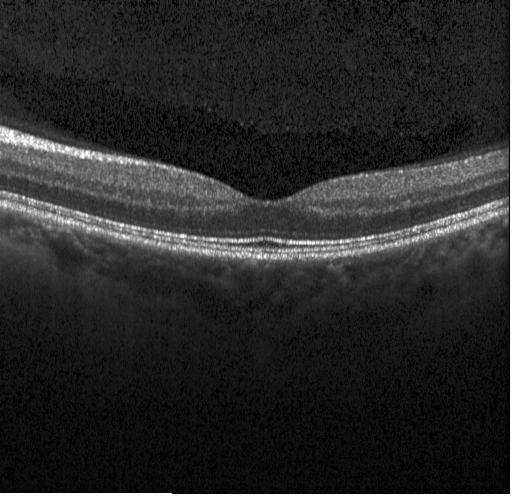

Spectral-domain OCT · instrument: Heidelberg Spectralis · fovea-centered · optical coherence tomography scan. Assessment: neither CNV, DME, nor drusen.